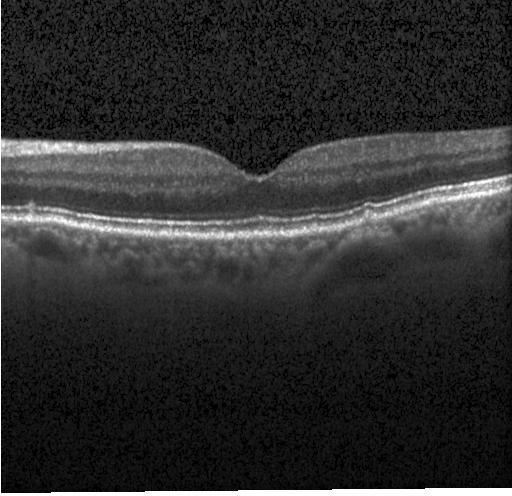

Macular OCT demonstrating multiple drusen.